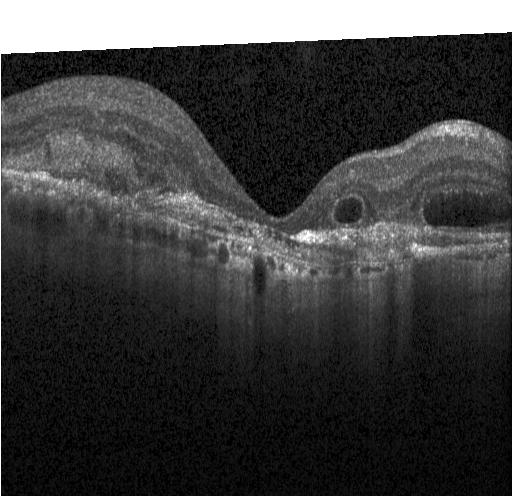

OCT finding: a choroidal neovascular membrane.